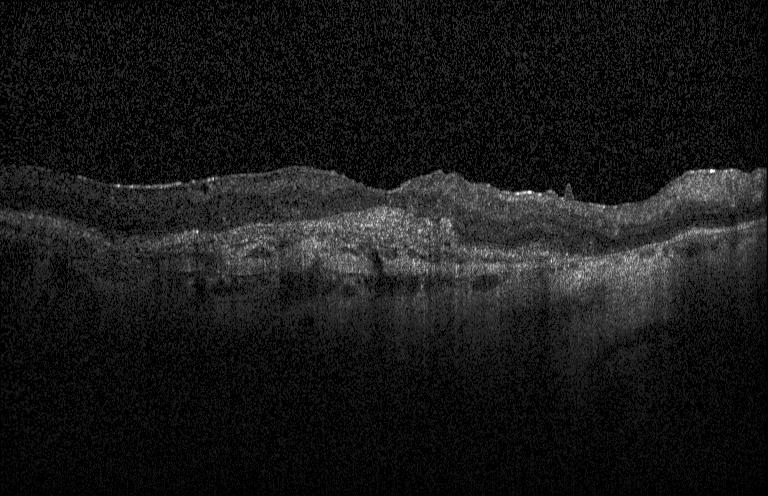 Macular OCT: a choroidal neovascular membrane.